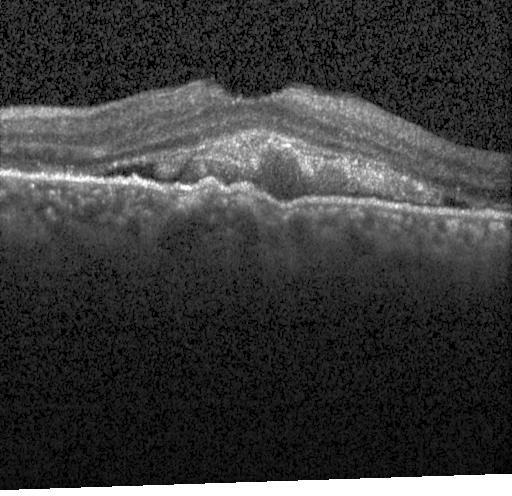 Acquired on a Heidelberg Spectralis, retinal OCT B-scan
Finding: a choroidal neovascular membrane.